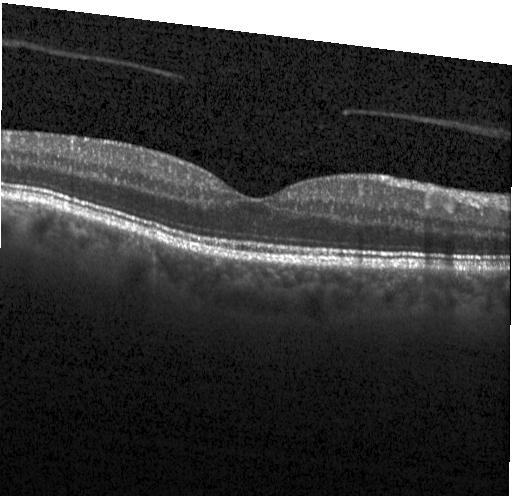 Acquired on a Heidelberg Spectralis. Spectral-domain OCT. Through the macula. Optical coherence tomography B-scan. Finding: no CNV, DME, or drusen.